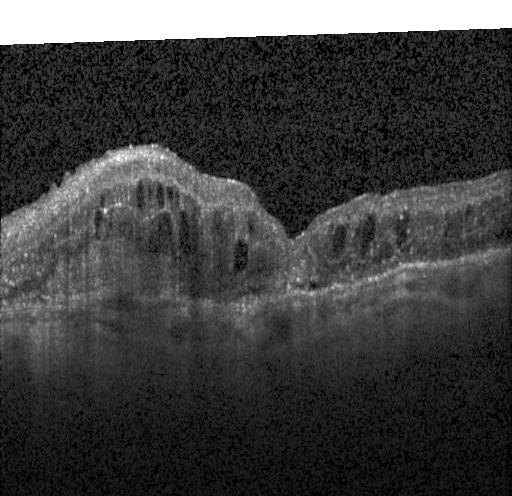
Spectral-domain optical coherence tomography. Fovea-centered. OCT B-scan.
Diagnosis: choroidal neovascularization (CNV).